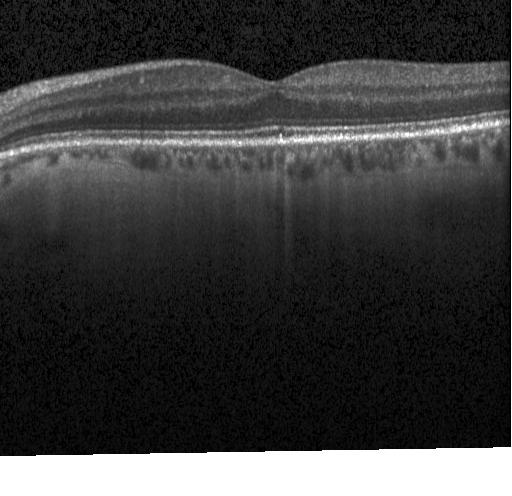

OCT finding: neither choroidal neovascularization, diabetic macular edema, nor drusen.